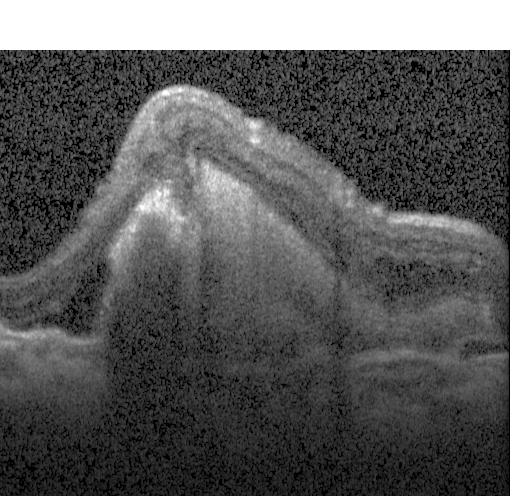
Dx: a choroidal neovascular membrane.